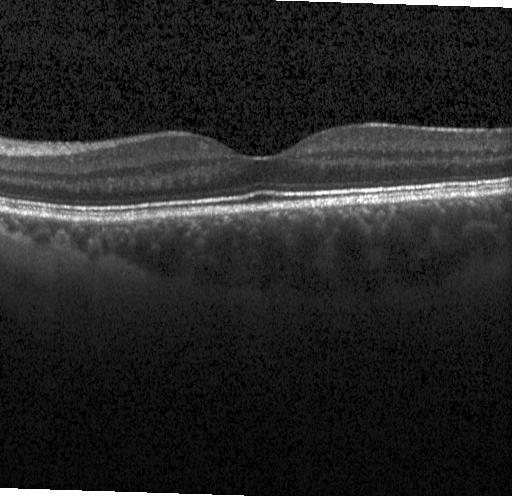 Instrument: Heidelberg Spectralis; through the macula; spectral-domain optical coherence tomography; optical coherence tomography scan. Impression: no choroidal neovascularization, no diabetic macular edema, and no drusen.